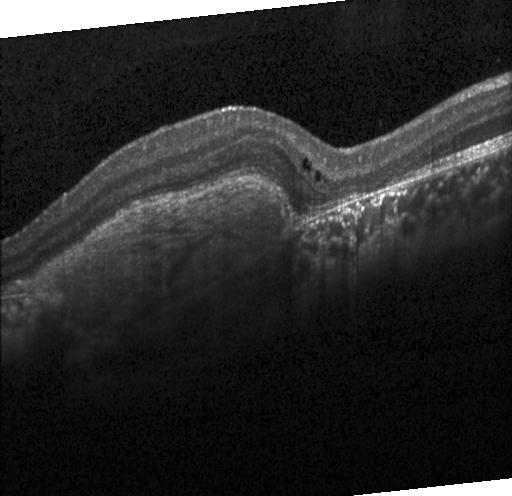
OCT finding: CNV.